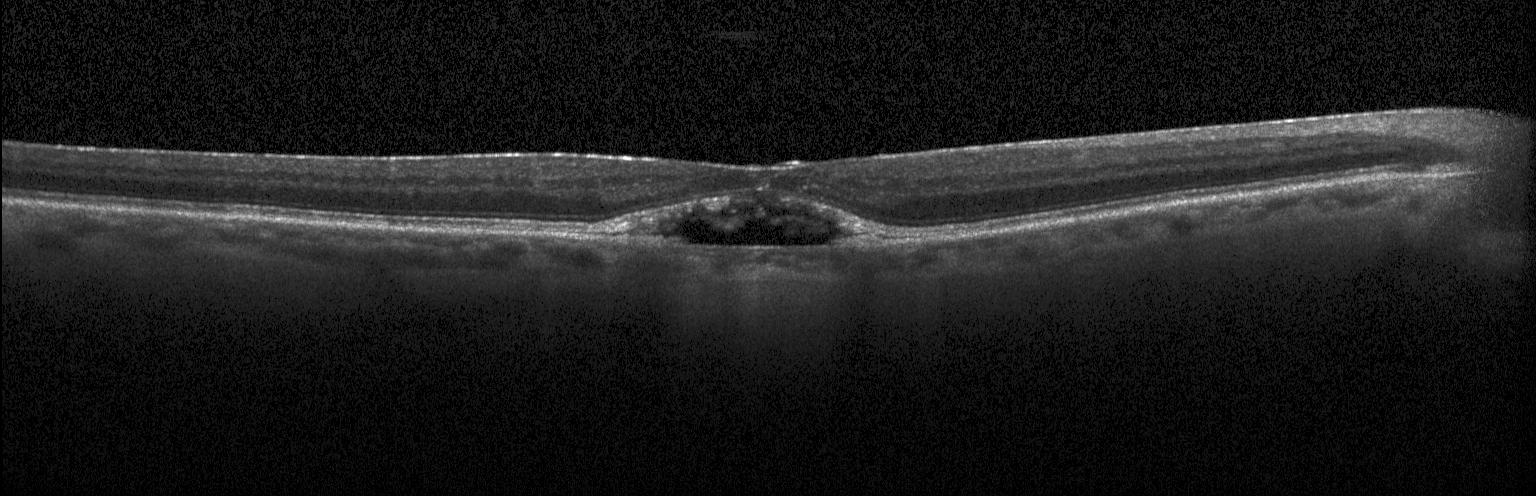
Heidelberg Spectralis OCT system; optical coherence tomography scan.
Impression: a choroidal neovascular membrane.